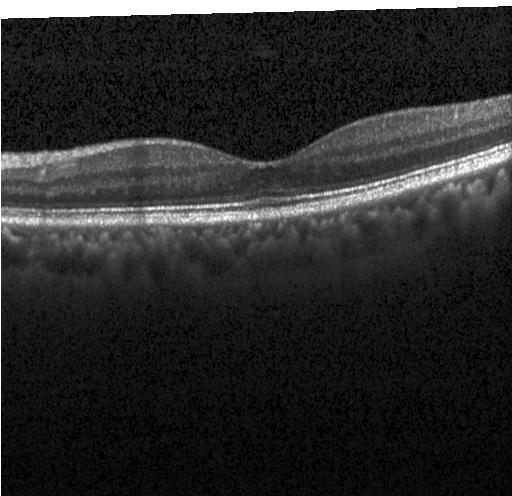

Horizontal scan through the fovea, OCT line scan, SD-OCT. Finding: no choroidal neovascularization, no diabetic macular edema, and no drusen.